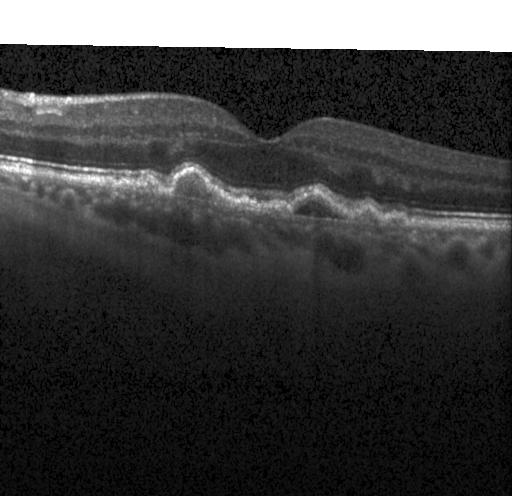

Instrument: Heidelberg Spectralis. SD-OCT. Fovea-centered. Optical coherence tomography B-scan — OCT finding: drusen.